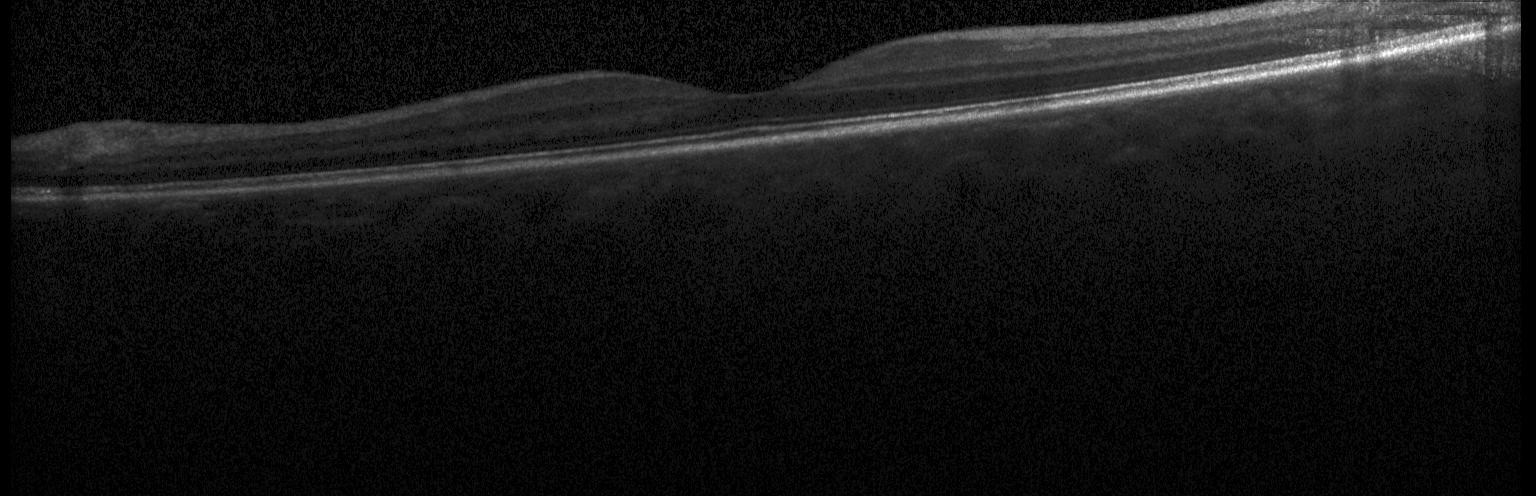

Heidelberg Spectralis, centered on the fovea, retinal OCT B-scan. Dx: neither CNV, DME, nor drusen.